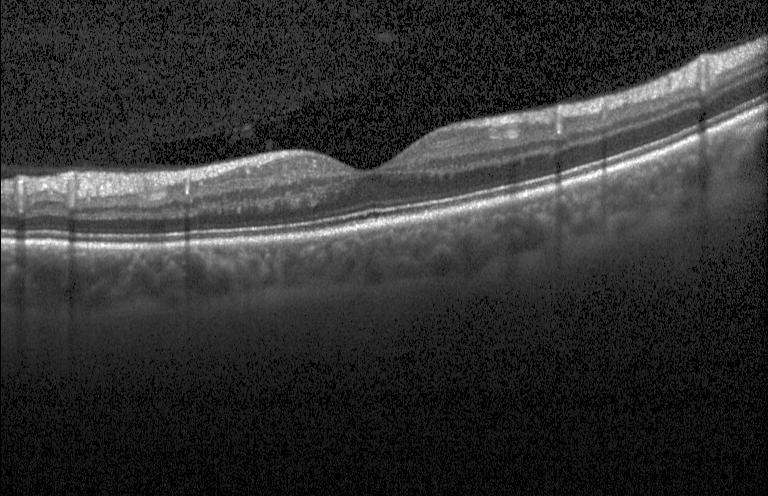

Finding: no choroidal neovascularization, diabetic macular edema, or drusen.